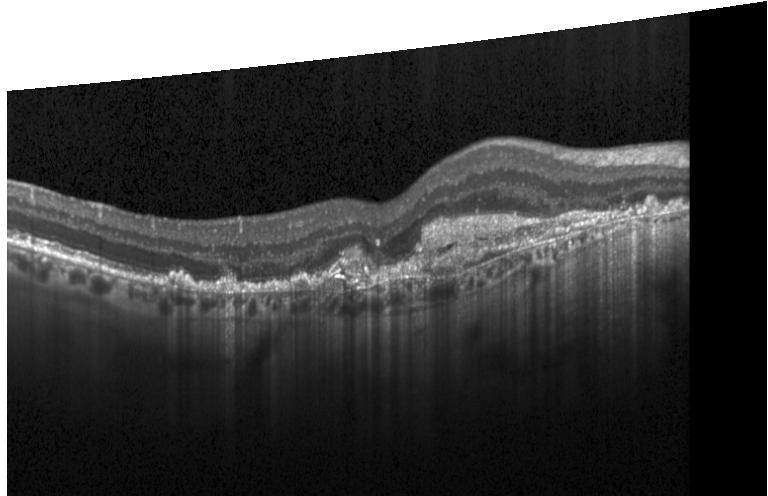

OCT line scan — Assessment: CNV.